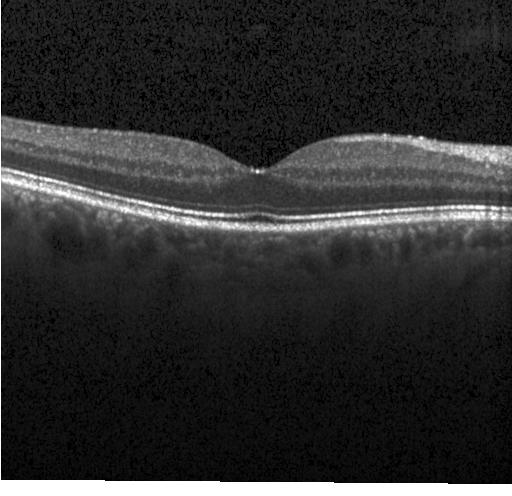
OCT B-scan.
No choroidal neovascularization, diabetic macular edema, or drusen.